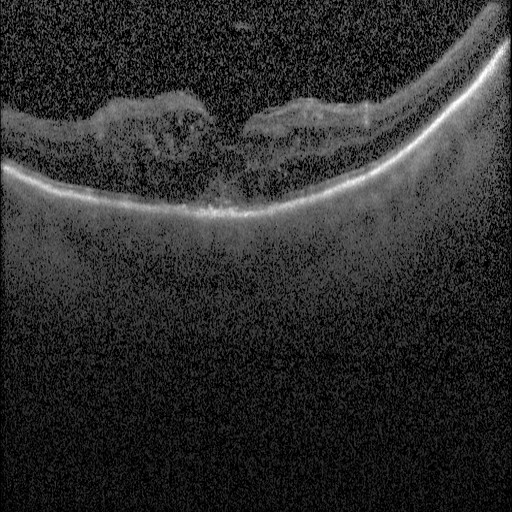
Macular scan, OCT B-scan
Macular OCT: diabetic macular edema.